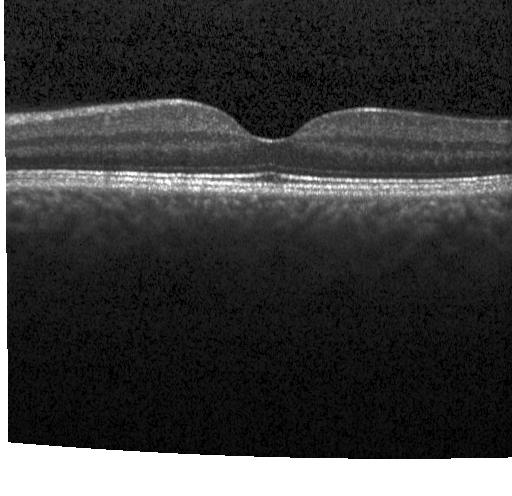

Optical coherence tomography B-scan; Heidelberg Spectralis; centered on the fovea
Macular OCT: no CNV, no DME, and no drusen.